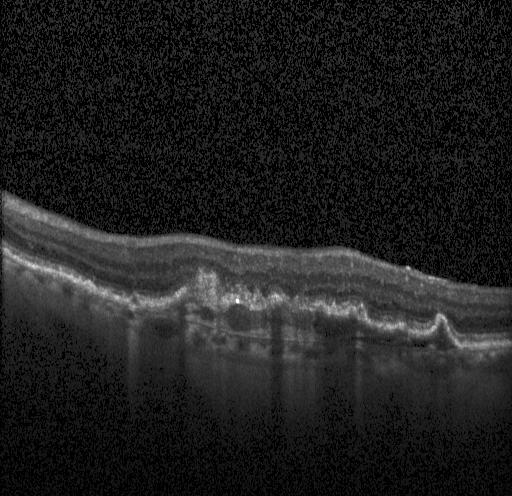
OCT line scan; instrument: Heidelberg Spectralis
Finding: a choroidal neovascular membrane.